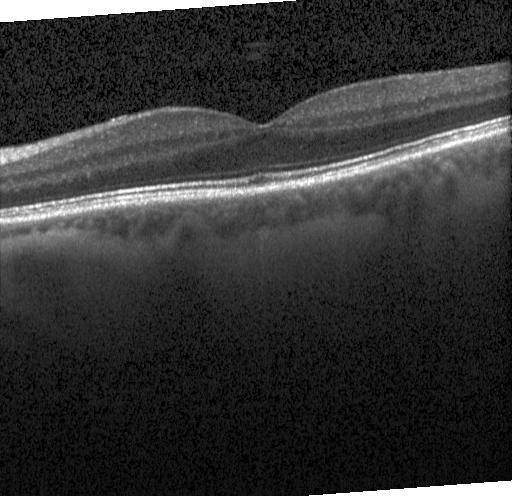 Horizontal scan through the fovea. Heidelberg Spectralis. OCT B-scan
Finding: no choroidal neovascularization, no diabetic macular edema, and no drusen.